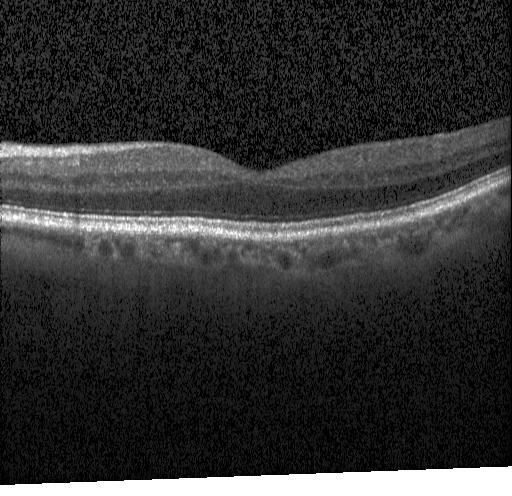
Spectral-domain OCT B-scan: no evidence of CNV, DME, or drusen.